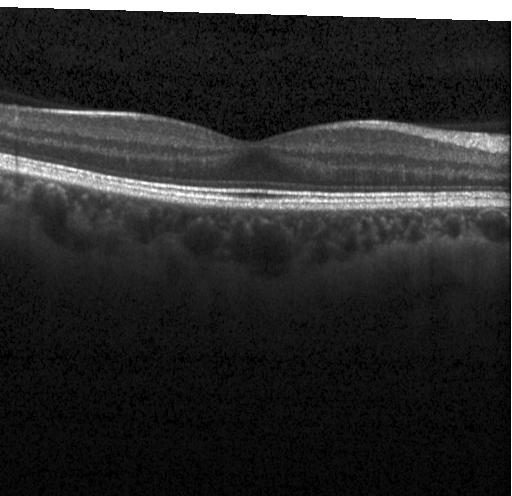

Retinal OCT cross-section showing no evidence of CNV, DME, or drusen.